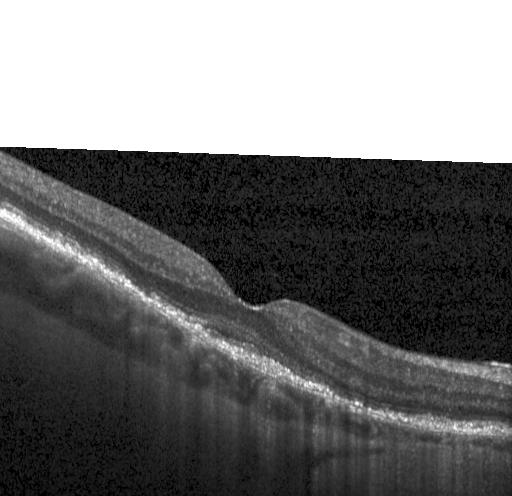

Dx: a choroidal neovascular membrane.